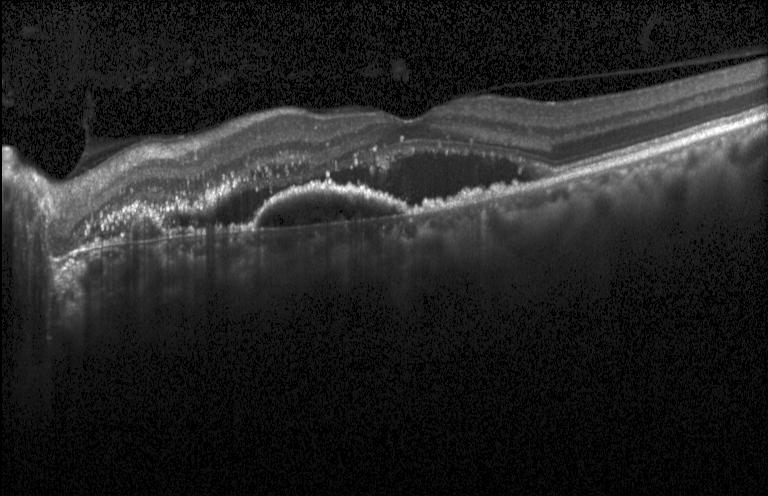
Spectral-domain OCT B-scan: choroidal neovascularization (CNV).